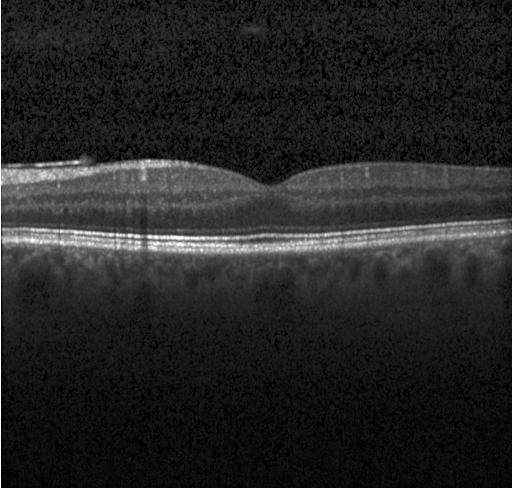
OCT line scan · horizontal scan through the fovea · SD-OCT · acquired on a Heidelberg Spectralis.
This B-scan demonstrates neither choroidal neovascularization, diabetic macular edema, nor drusen.